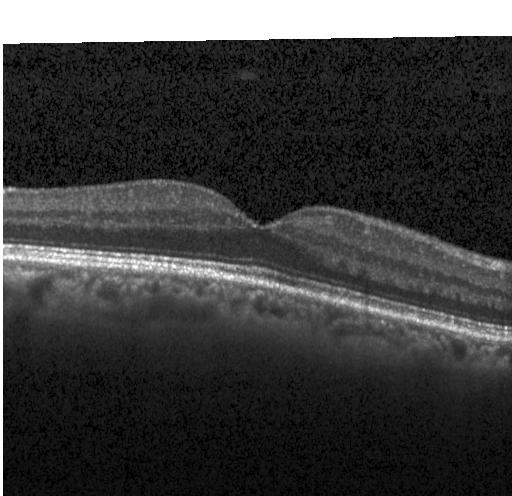
Retinal OCT B-scan. Spectral-domain optical coherence tomography. OCT finding: no choroidal neovascularization, diabetic macular edema, or drusen.